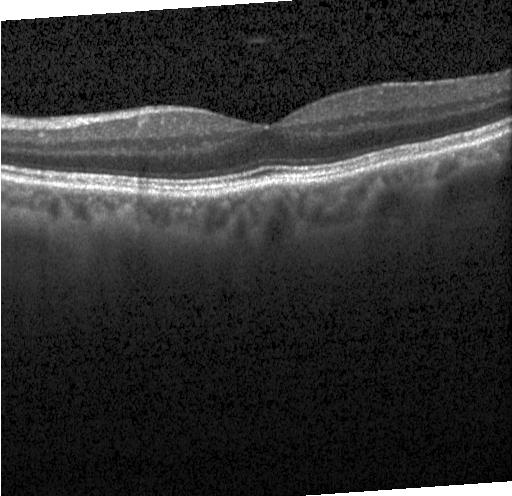

Diagnosis: no evidence of choroidal neovascularization, diabetic macular edema, or drusen.